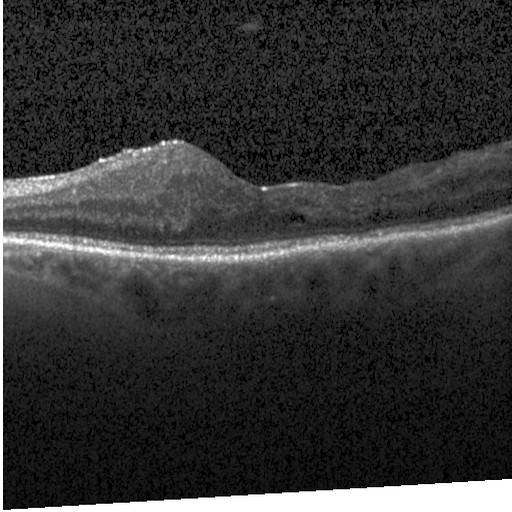

The scan shows diabetic macular edema.